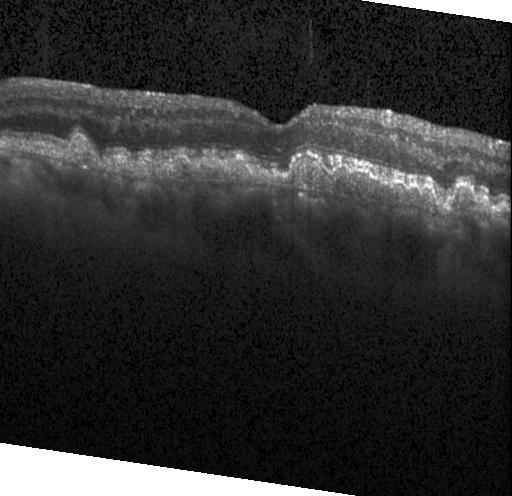 Retinal OCT B-scan, SD-OCT.
Impression: CNV.